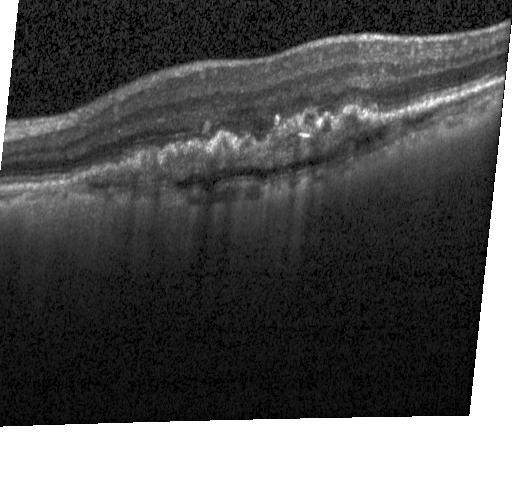

OCT line scan. The scan shows choroidal neovascularization.